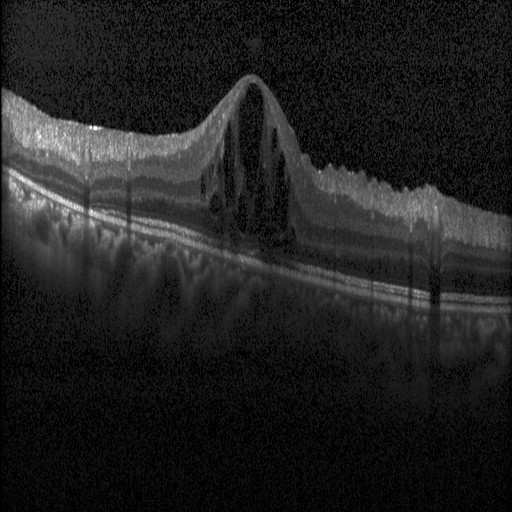

Fovea-centered. Acquired on a Heidelberg Spectralis. Spectral-domain OCT. OCT line scan.
Diagnosis: DME.